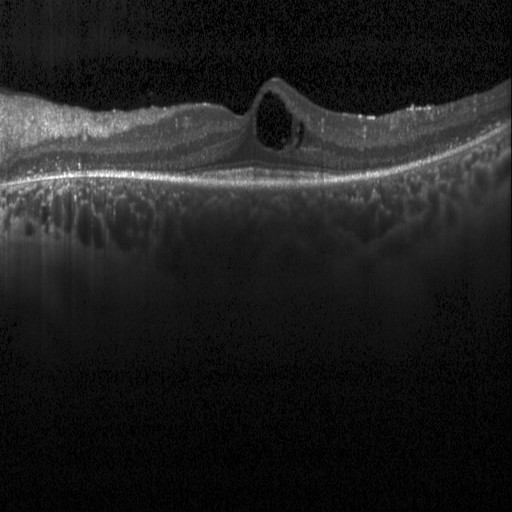

Retinal OCT B-scan. Horizontal scan through the fovea. Acquired on a Heidelberg Spectralis
DME.